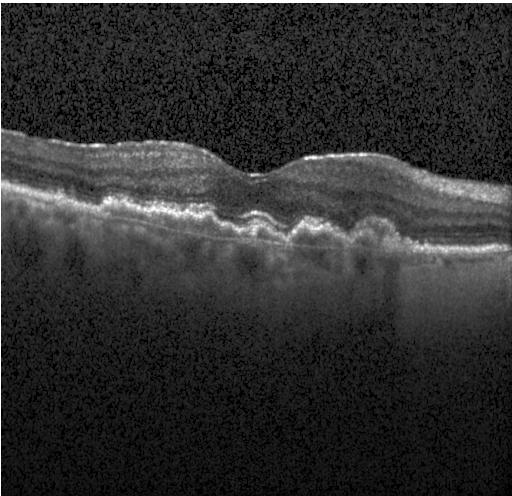 Diagnosis: a choroidal neovascular membrane.